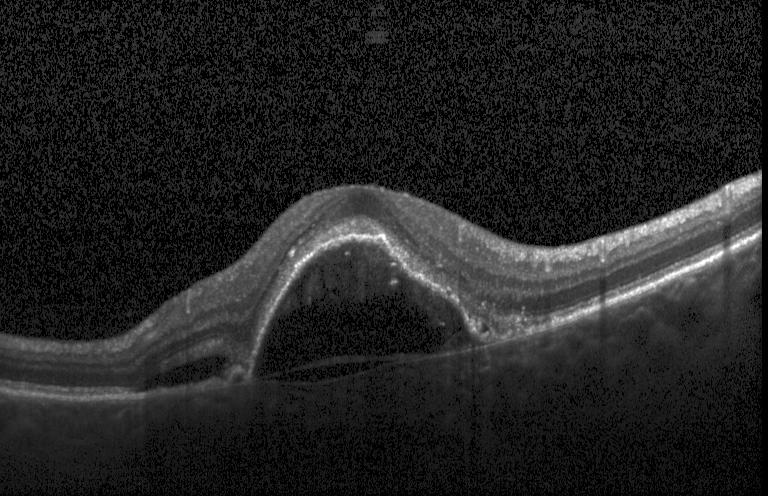
Macular OCT demonstrating a choroidal neovascular membrane.